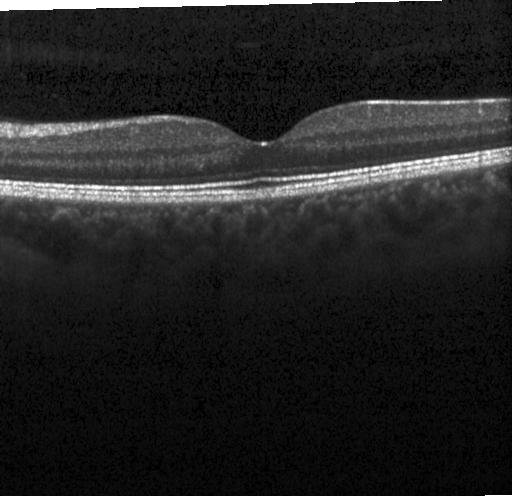 Diagnosis: no evidence of choroidal neovascularization, diabetic macular edema, or drusen.